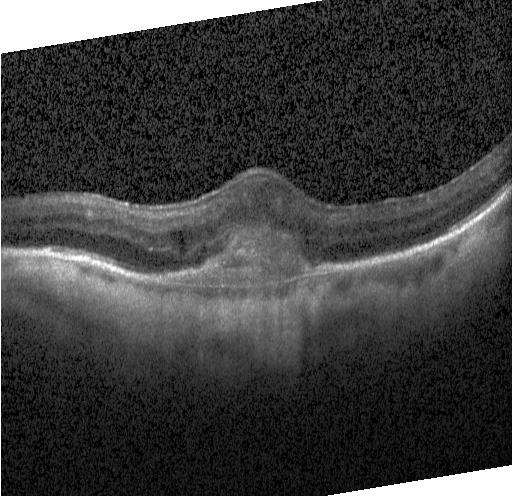

OCT B-scan; acquired on a Heidelberg Spectralis; horizontal scan through the fovea. Dx: choroidal neovascularization.